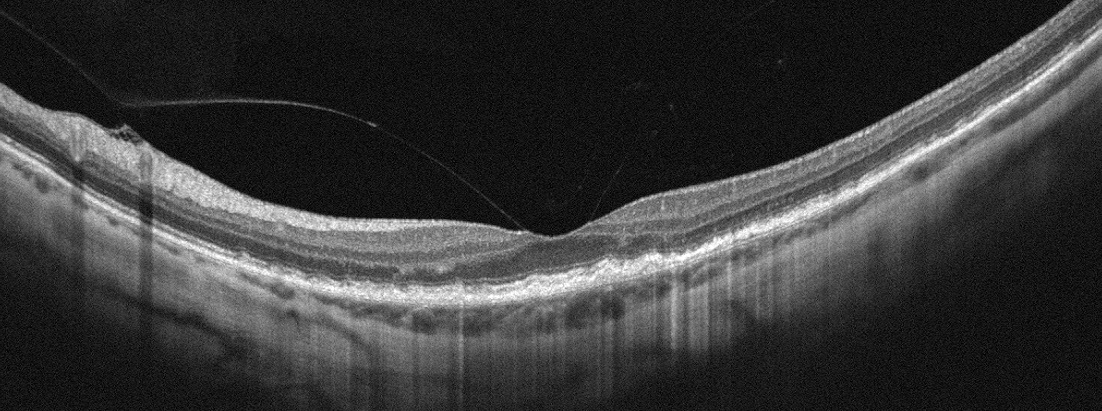

Optovue Avanti RTVue XR. Retinal OCT B-scan
Impression: age-related macular degeneration (AMD).